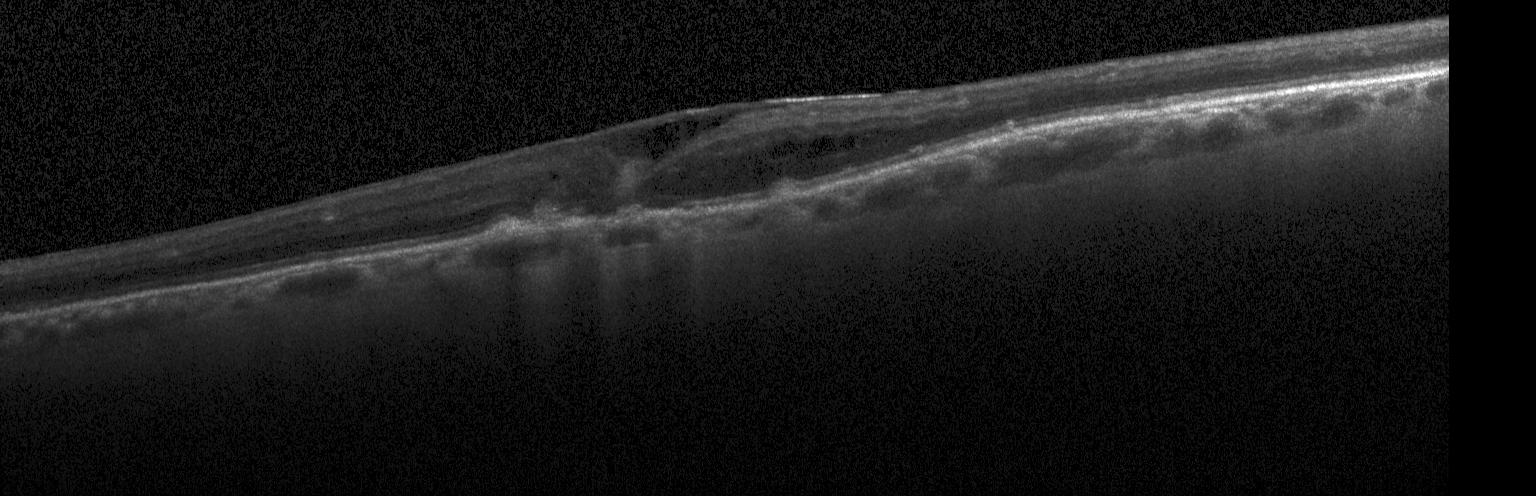

Centered on the fovea; instrument: Heidelberg Spectralis; optical coherence tomography scan — Diagnosis: choroidal neovascularization (CNV).